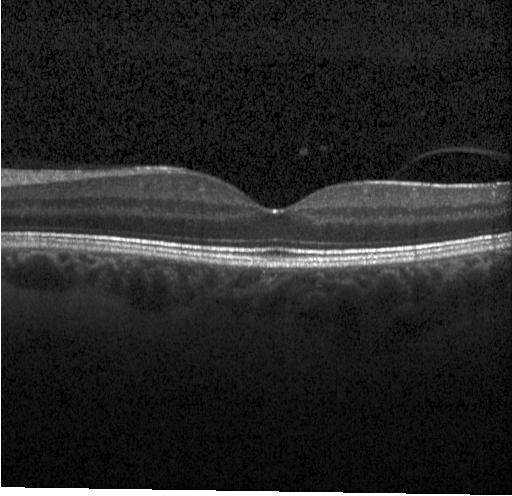 This B-scan demonstrates neither choroidal neovascularization, diabetic macular edema, nor drusen.